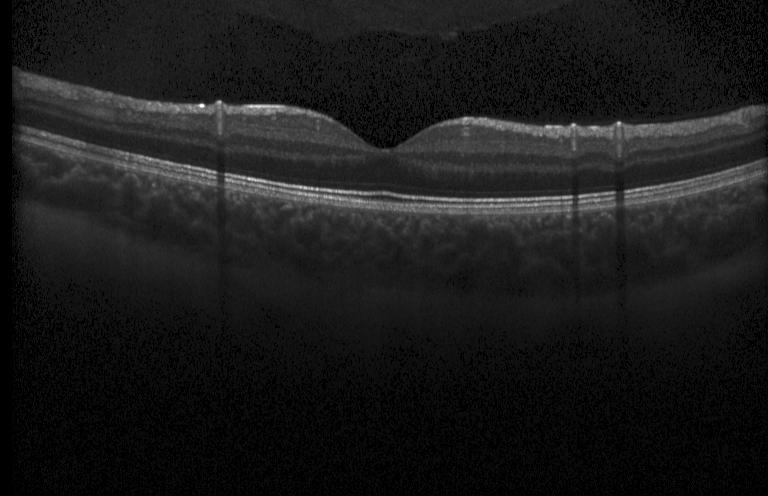
SD-OCT · optical coherence tomography scan · centered on the fovea. Finding: neither choroidal neovascularization, diabetic macular edema, nor drusen.